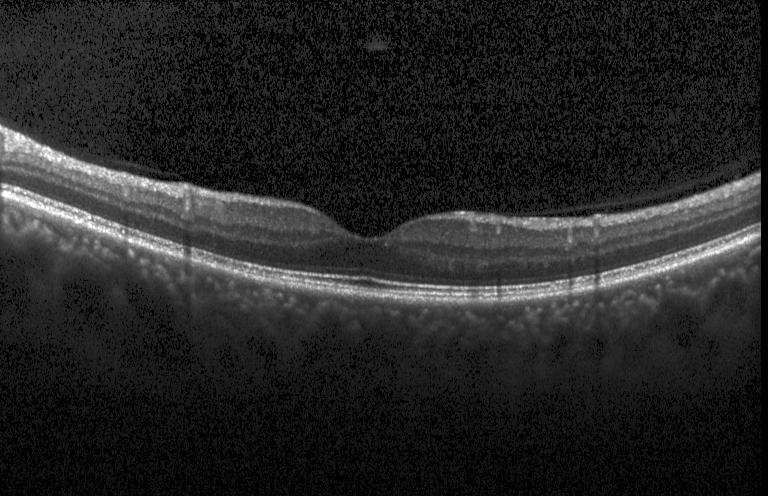 Spectral-domain optical coherence tomography; OCT B-scan.
This B-scan demonstrates no evidence of choroidal neovascularization, diabetic macular edema, or drusen.